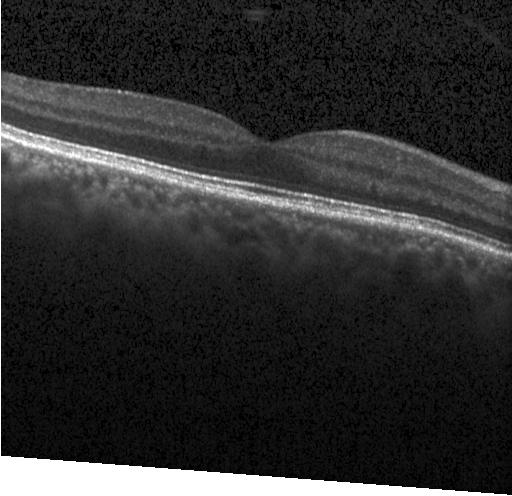

Diagnosis: neither CNV, DME, nor drusen.